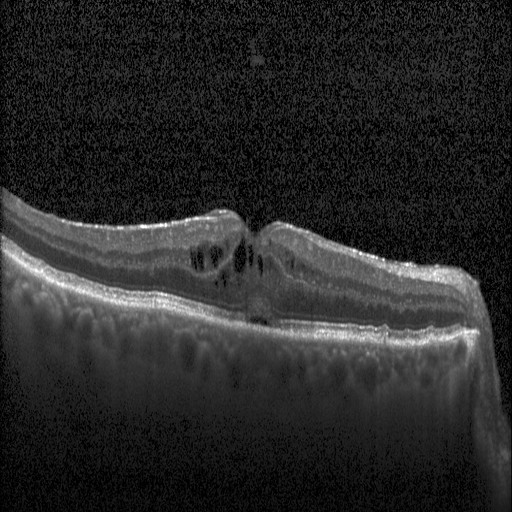
Macular OCT: DME.